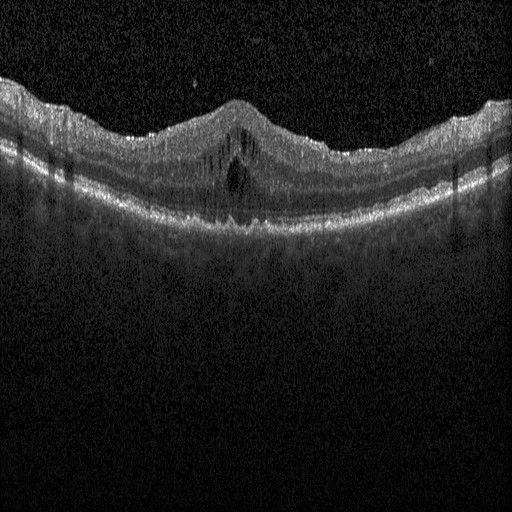

Instrument: Heidelberg Spectralis, OCT line scan, spectral-domain OCT.
The scan shows DME.